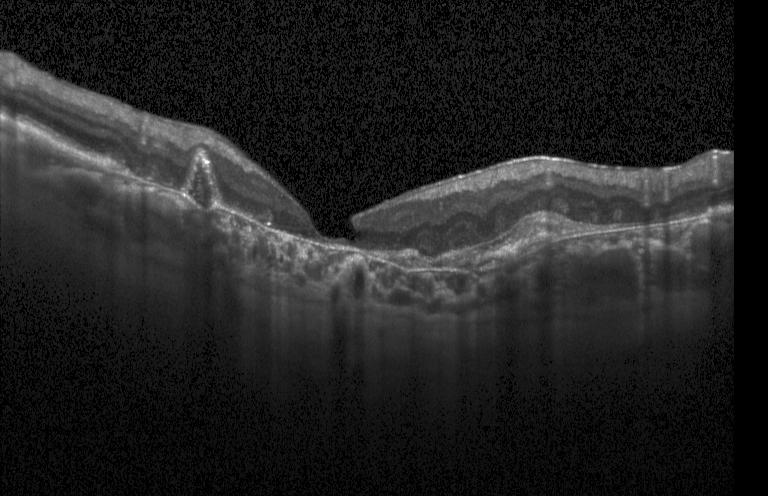 Optical coherence tomography B-scan. Spectral-domain OCT. Heidelberg Spectralis — Diagnosis: a choroidal neovascular membrane.